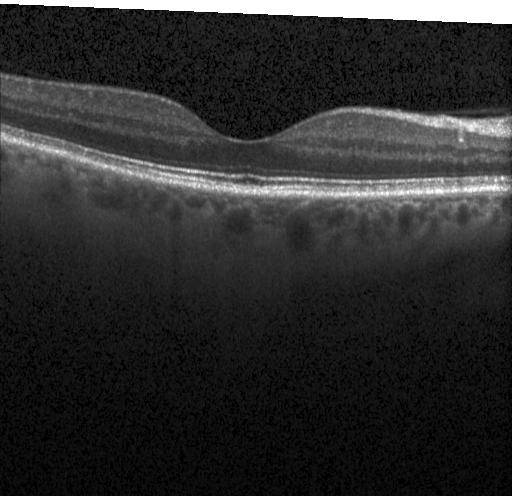

The scan shows no choroidal neovascularization, no diabetic macular edema, and no drusen.